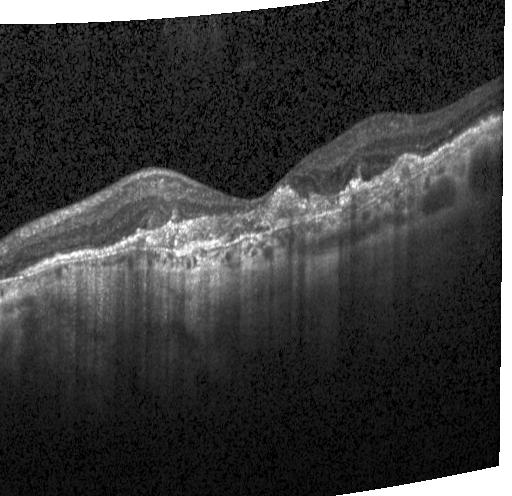

Diagnosis: a choroidal neovascular membrane.